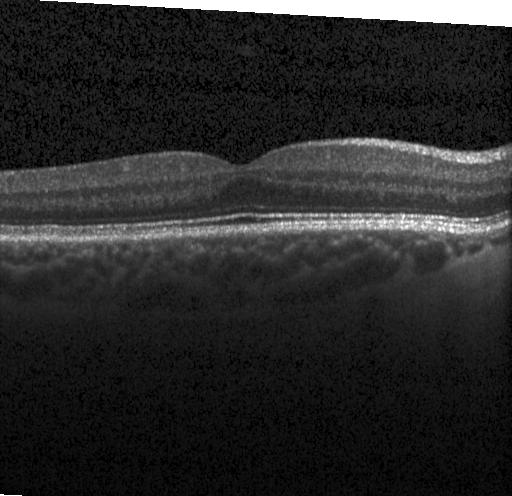
Heidelberg Spectralis OCT system. Optical coherence tomography B-scan. Fovea-centered. Assessment: no choroidal neovascularization, no diabetic macular edema, and no drusen.